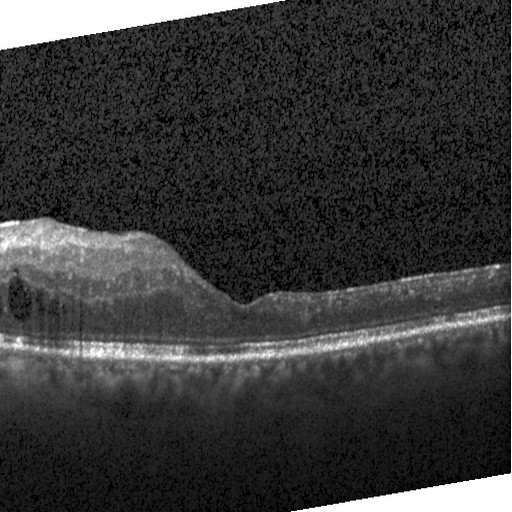 Retinal OCT cross-section showing diabetic macular edema.